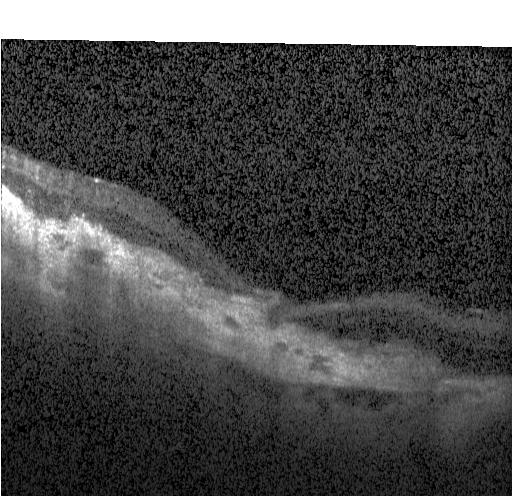

Retinal OCT B-scan.
Finding: a choroidal neovascular membrane.